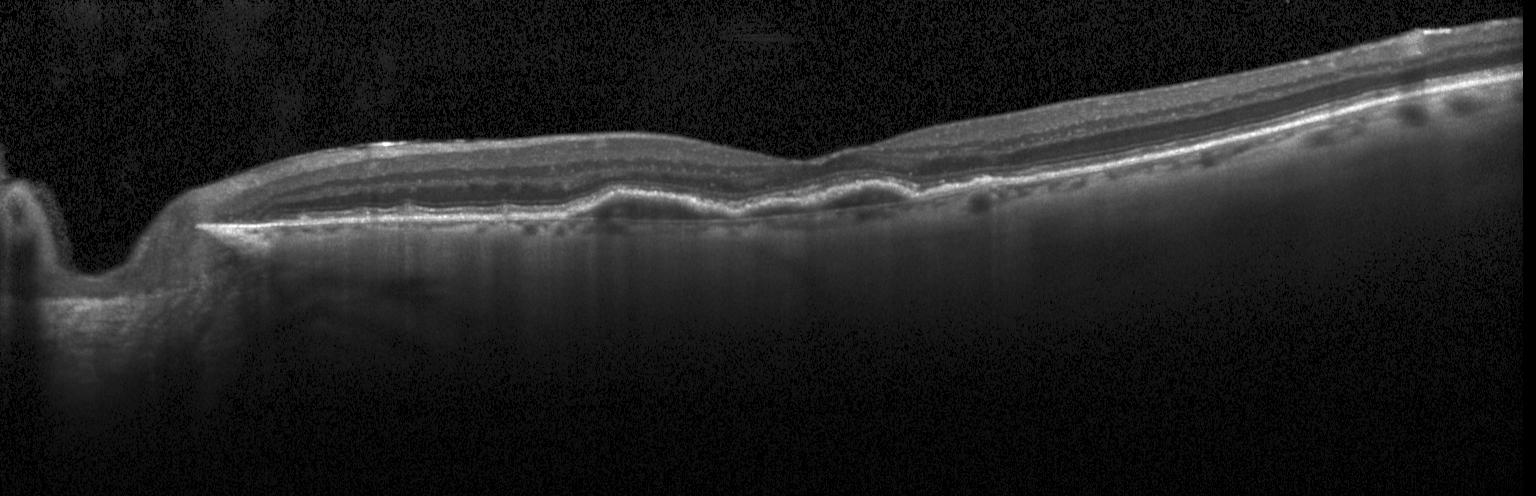

Spectral-domain optical coherence tomography, retinal OCT B-scan, instrument: Heidelberg Spectralis, fovea-centered. Dx: choroidal neovascularization.